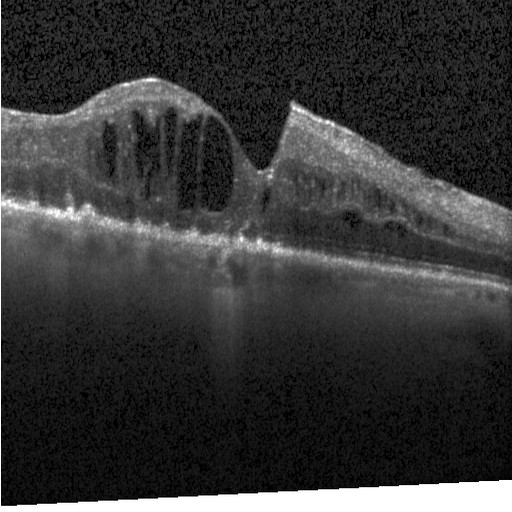
Diagnosis: DME.